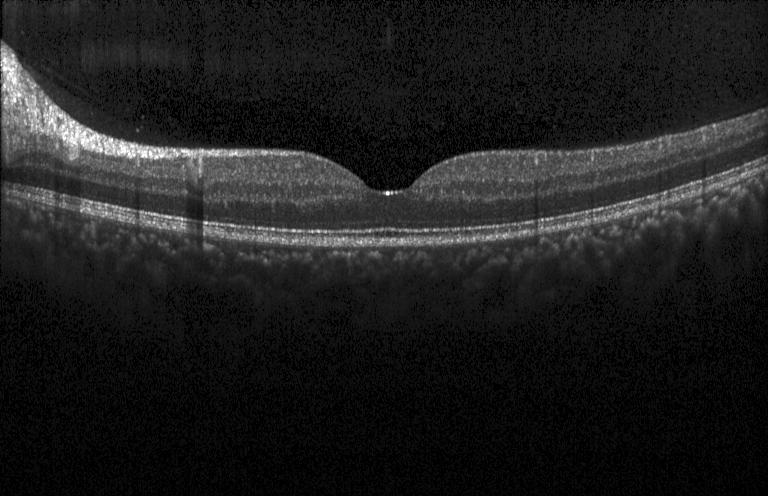

Retinal OCT cross-section; spectral-domain OCT; macular scan; Heidelberg Spectralis OCT system. Impression: neither choroidal neovascularization, diabetic macular edema, nor drusen.